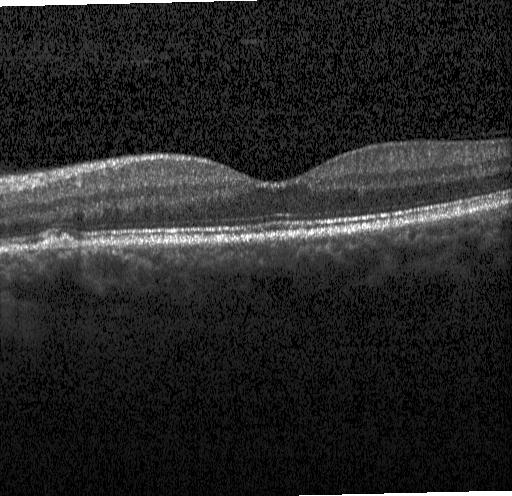 Dx: drusen.